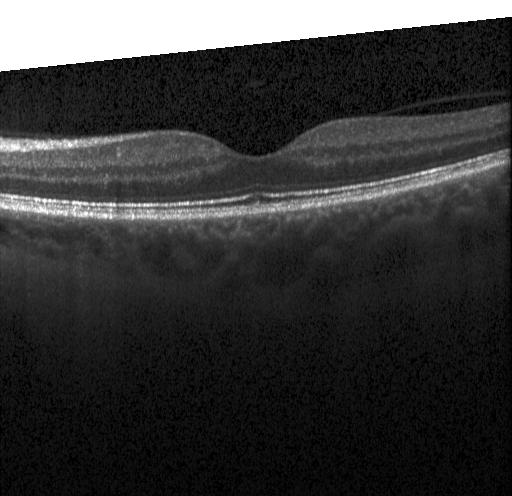
Impression: neither CNV, DME, nor drusen.